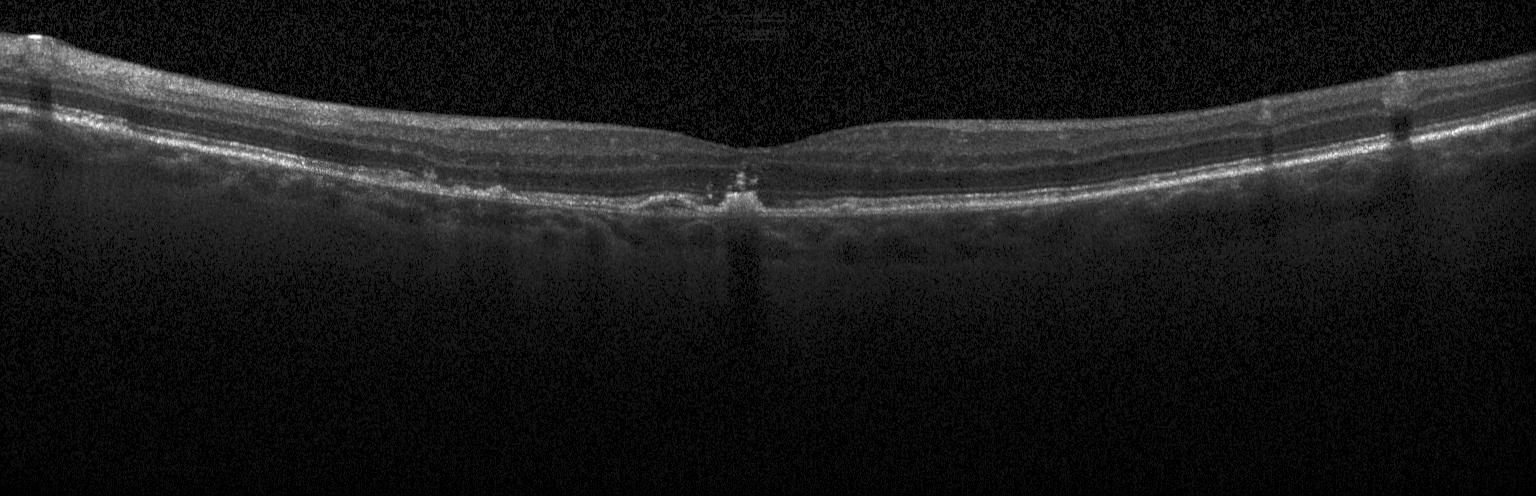 OCT B-scan.
The scan shows choroidal neovascularization.